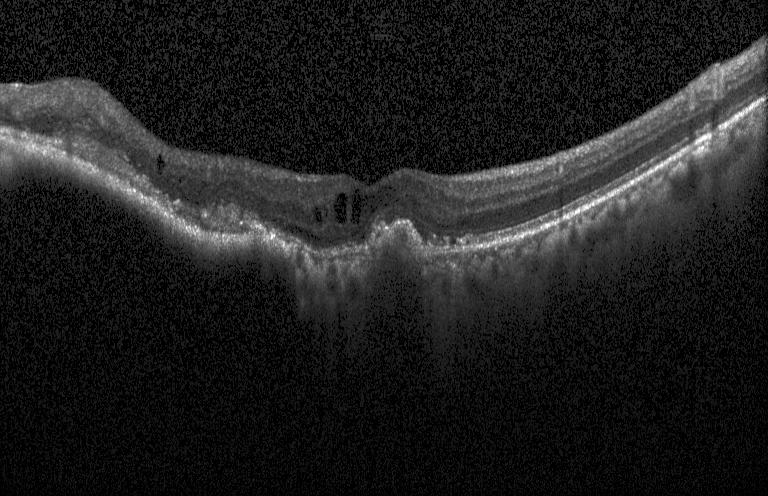
Through the macula, Heidelberg Spectralis OCT system, optical coherence tomography B-scan, SD-OCT
Assessment: choroidal neovascularization.